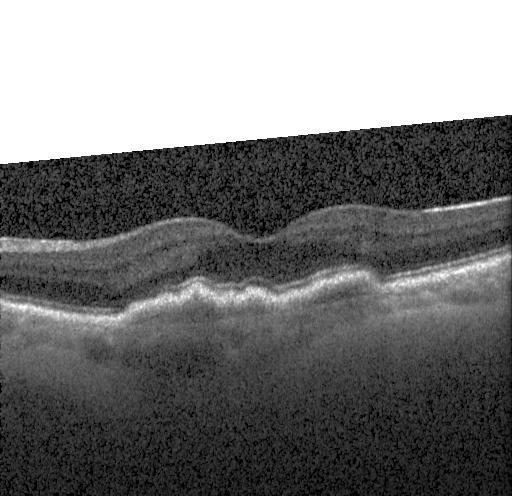 Retinal OCT B-scan. Impression: a choroidal neovascular membrane.